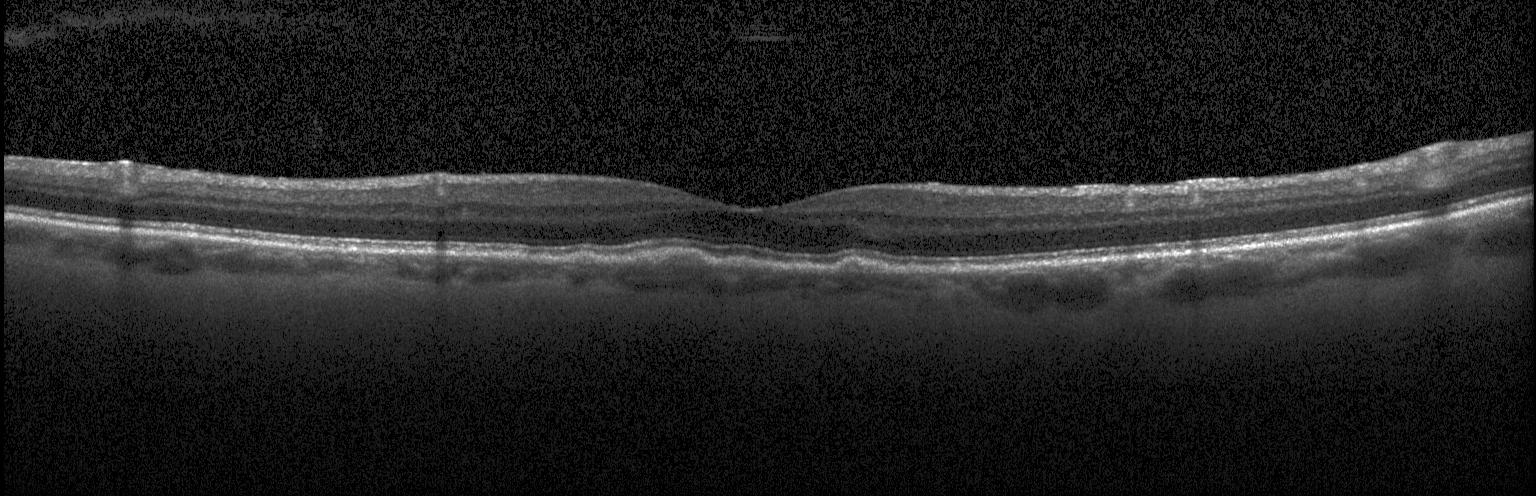
Spectral-domain OCT. Instrument: Heidelberg Spectralis. OCT line scan.
Finding: multiple drusen.